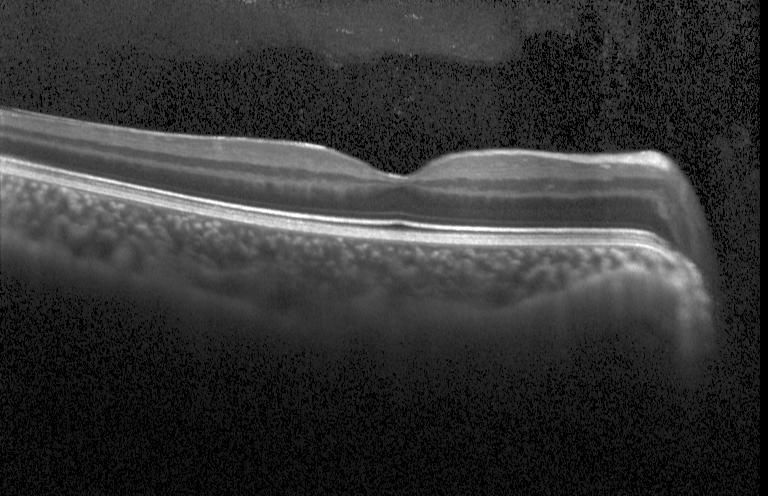

Spectral-domain OCT B-scan: no evidence of choroidal neovascularization, diabetic macular edema, or drusen.